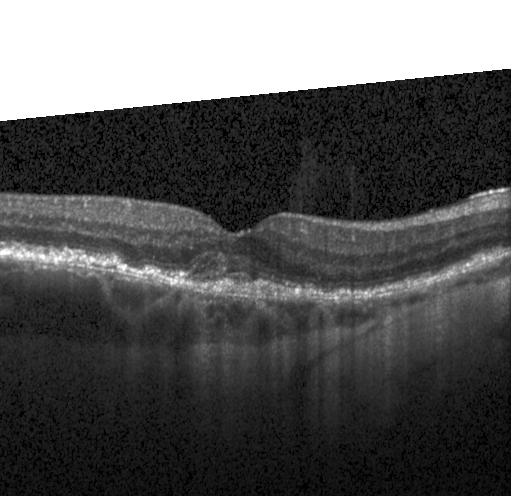
Macular OCT demonstrating choroidal neovascularization (CNV).